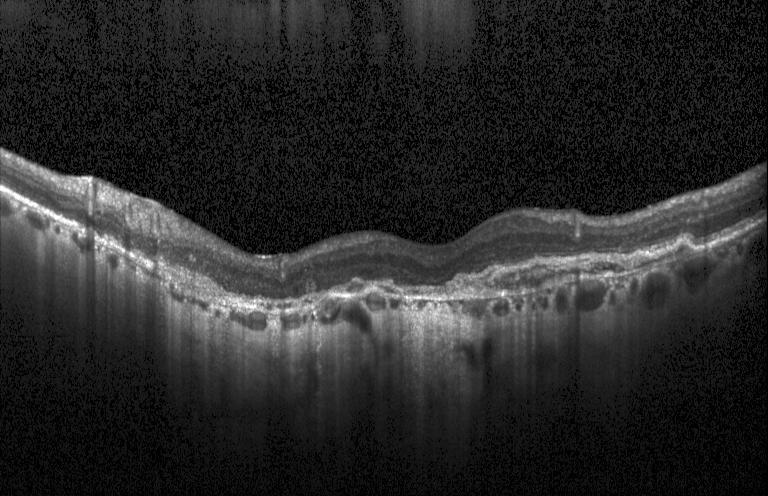
Macular OCT: choroidal neovascularization.